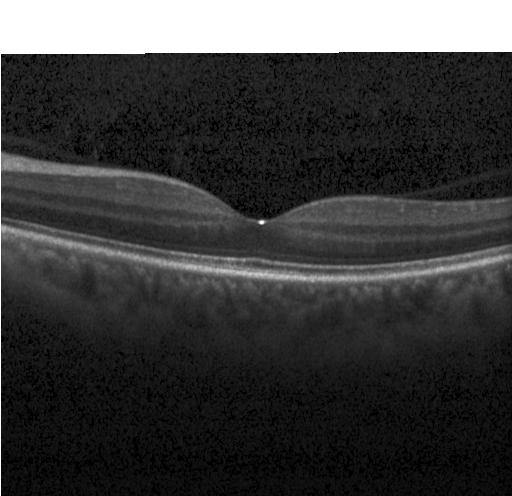

Optical coherence tomography B-scan
OCT finding: no CNV, no DME, and no drusen.